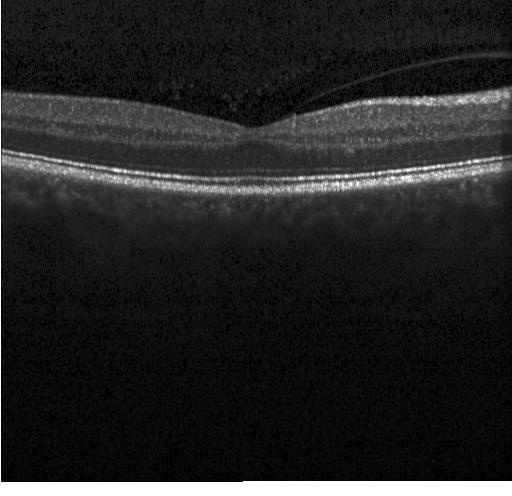
Finding: no CNV, DME, or drusen.